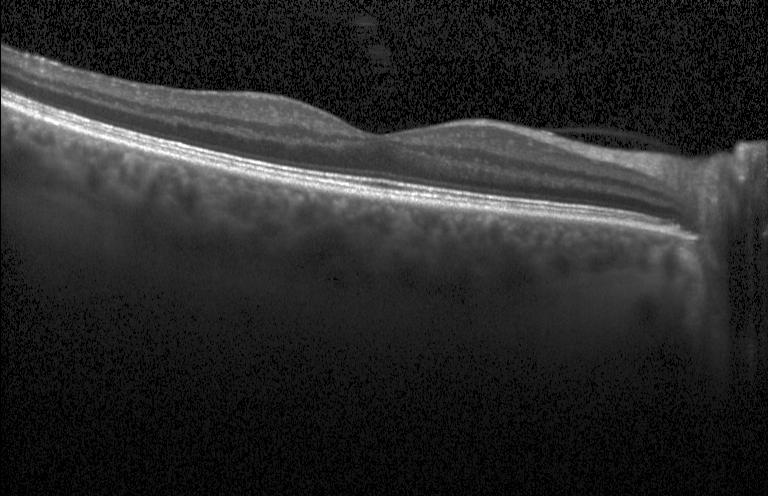

Spectral-domain optical coherence tomography · OCT B-scan
Diagnosis: neither choroidal neovascularization, diabetic macular edema, nor drusen.